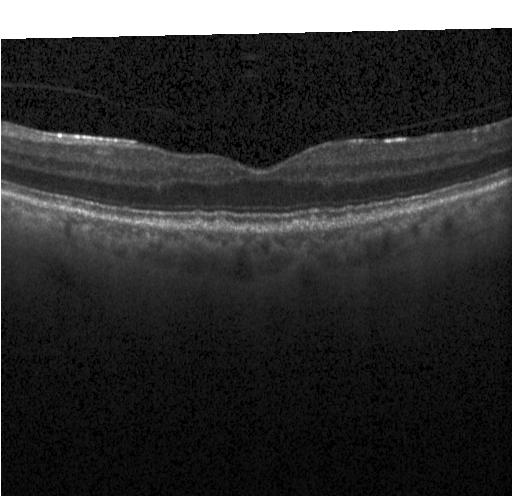

OCT B-scan showing sub-RPE drusenoid deposits.